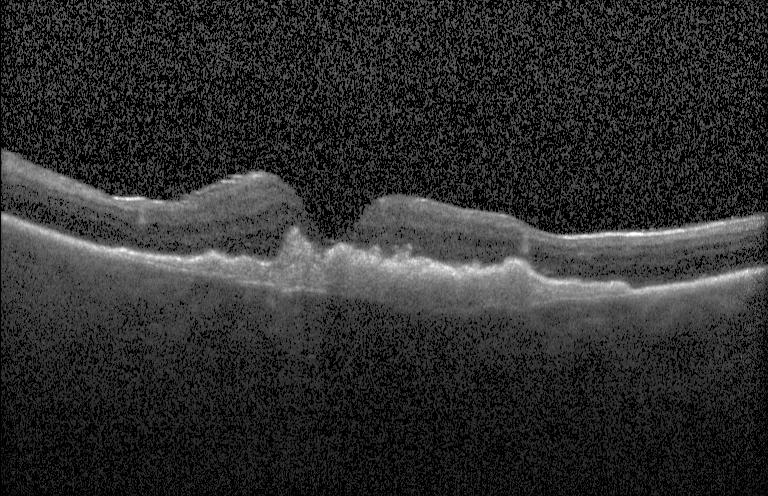 Macular scan · OCT B-scan · instrument: Heidelberg Spectralis · spectral-domain OCT. Finding: choroidal neovascularization.